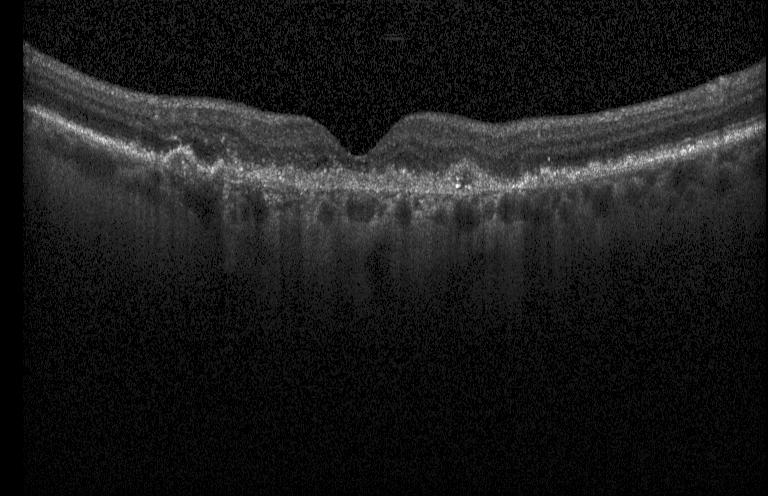

OCT B-scan — OCT finding: choroidal neovascularization (CNV).